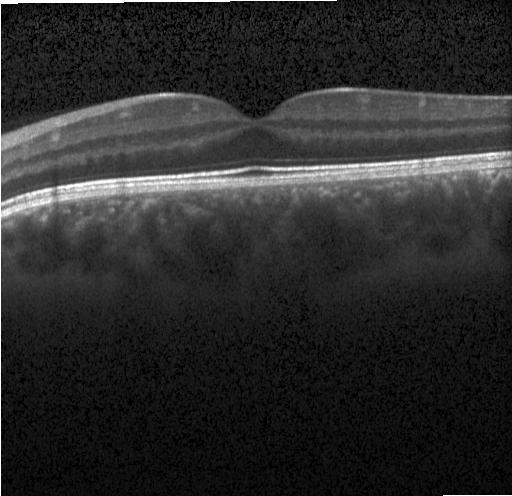 Optical coherence tomography scan · acquired on a Heidelberg Spectralis · SD-OCT.
Finding: neither choroidal neovascularization, diabetic macular edema, nor drusen.